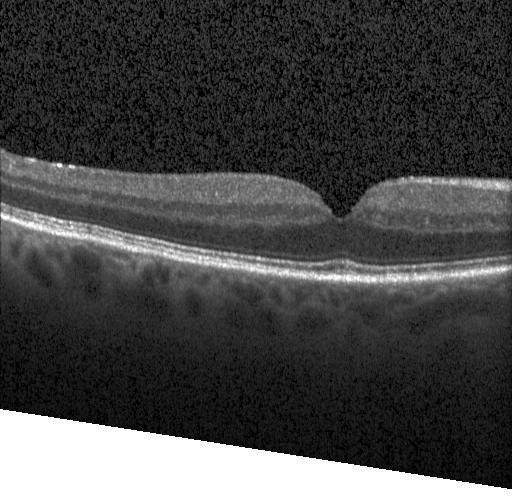 Macular OCT demonstrating no CNV, DME, or drusen.